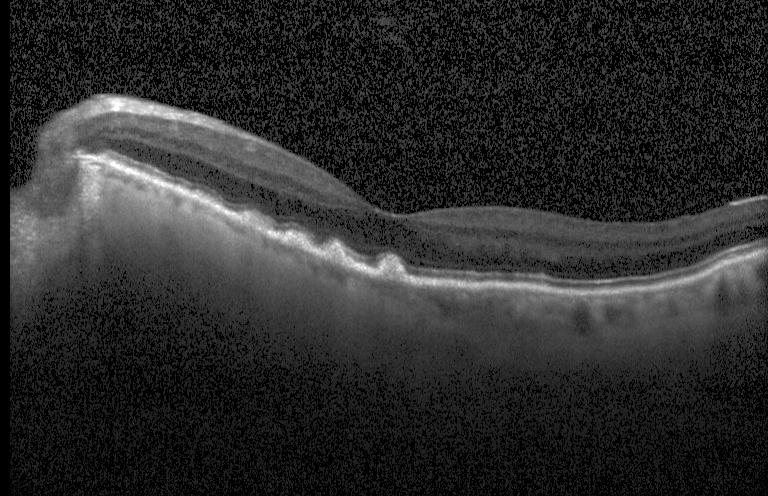
Optical coherence tomography B-scan; instrument: Heidelberg Spectralis; centered on the fovea; SD-OCT. Finding: drusen.